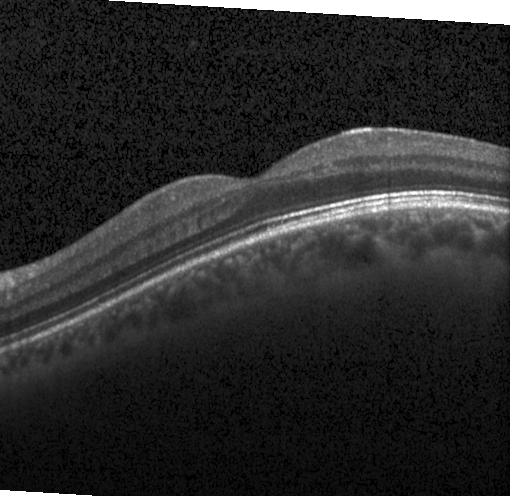 Optical coherence tomography scan.
This B-scan demonstrates no CNV, no DME, and no drusen.